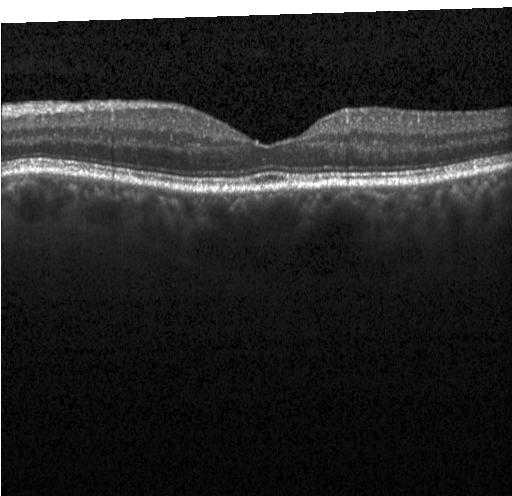

This B-scan demonstrates no evidence of choroidal neovascularization, diabetic macular edema, or drusen.